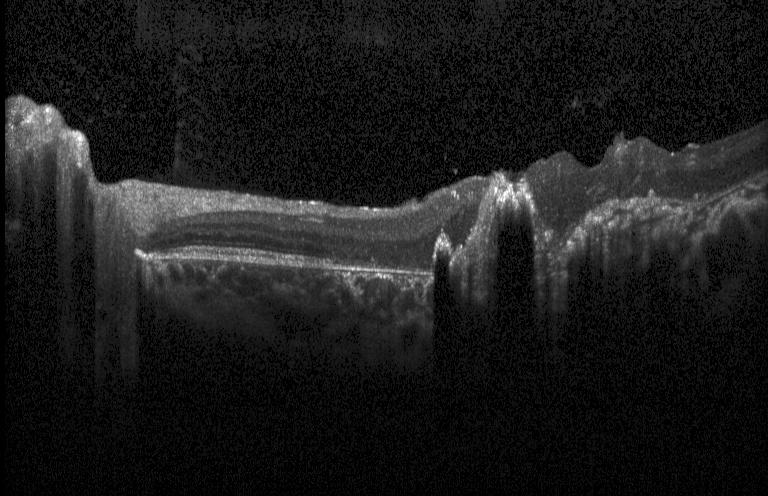
Optical coherence tomography B-scan
Finding: a choroidal neovascular membrane.